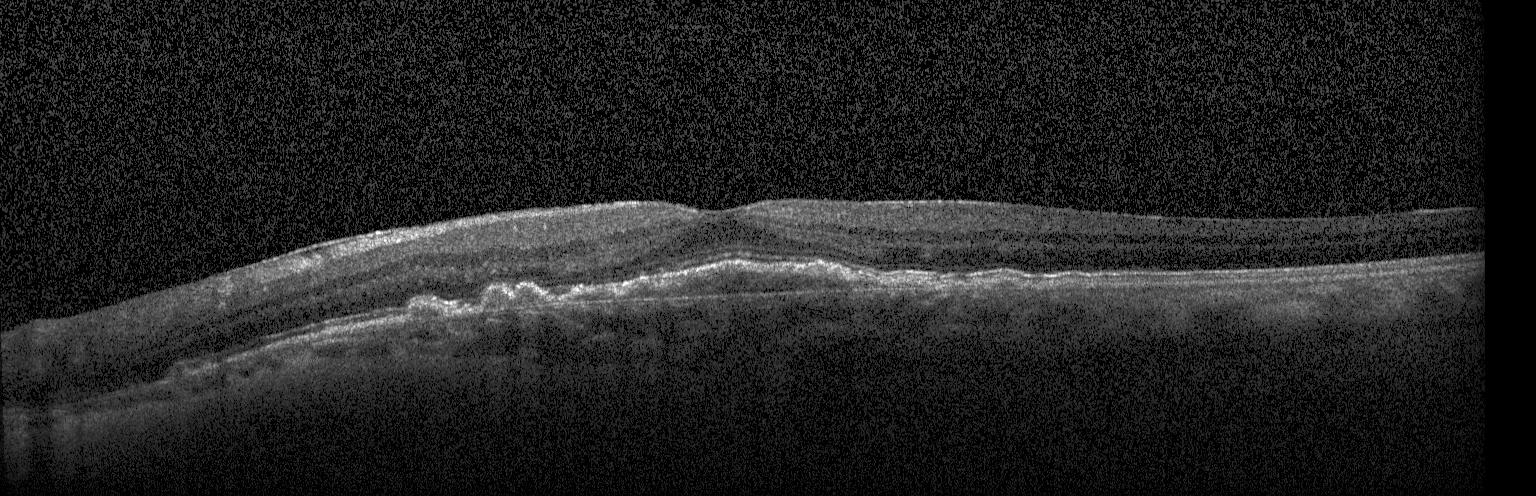 OCT B-scan. Spectral-domain OCT. Instrument: Heidelberg Spectralis — Assessment: a choroidal neovascular membrane.